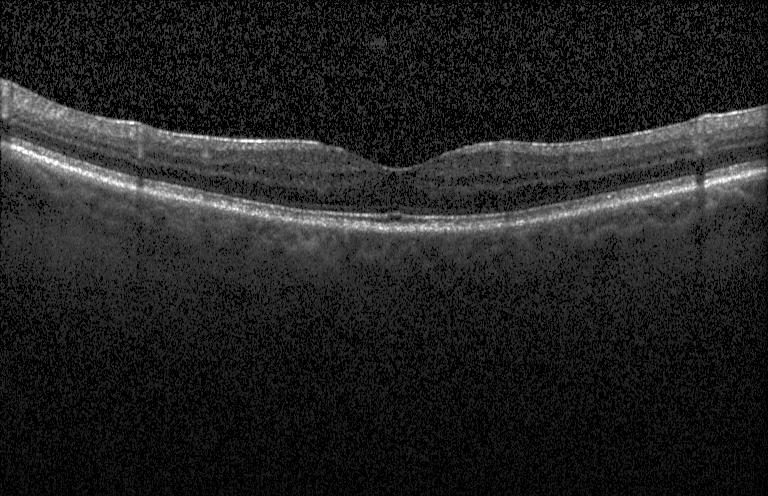
Heidelberg Spectralis, spectral-domain optical coherence tomography, retinal OCT cross-section. Macular OCT: neither choroidal neovascularization, diabetic macular edema, nor drusen.